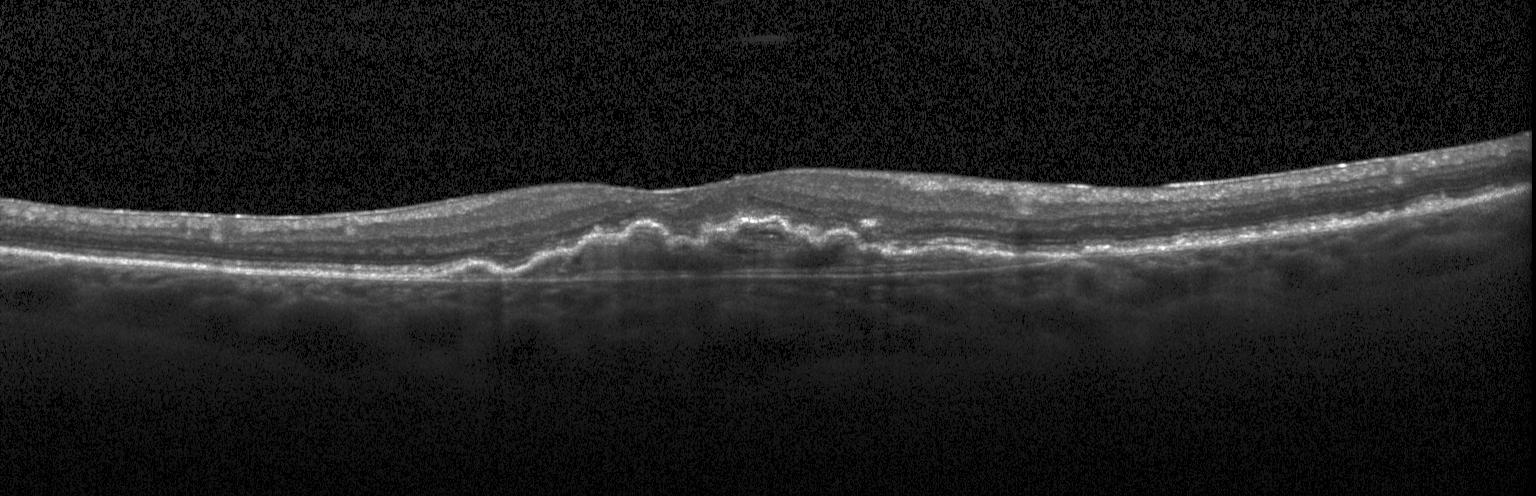

Fovea-centered. Optical coherence tomography scan. Diagnosis: a choroidal neovascular membrane.